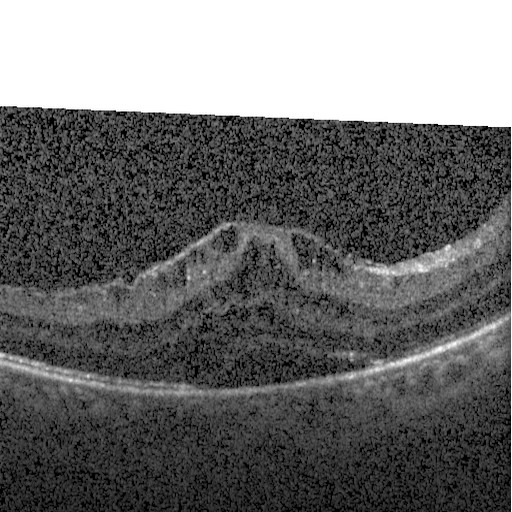

OCT B-scan. Spectral-domain OCT. Macular scan — Diabetic macular edema (DME).